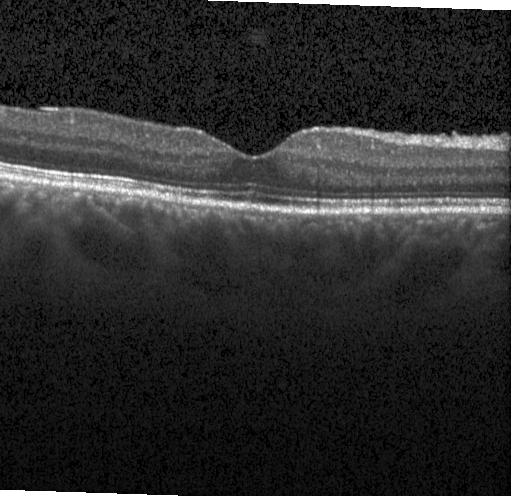

Retinal OCT B-scan.
Diagnosis: no choroidal neovascularization, no diabetic macular edema, and no drusen.